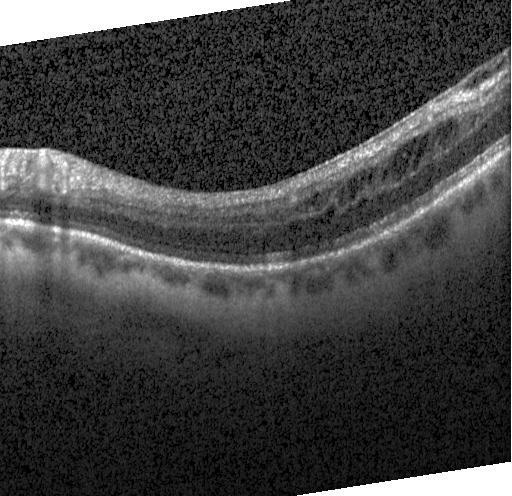 Optical coherence tomography scan.
Diagnosis: DME.